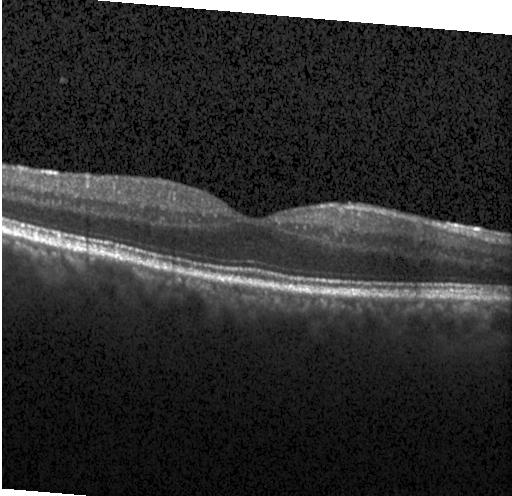 Through the macula, Heidelberg Spectralis OCT system, optical coherence tomography scan
No choroidal neovascularization, diabetic macular edema, or drusen.